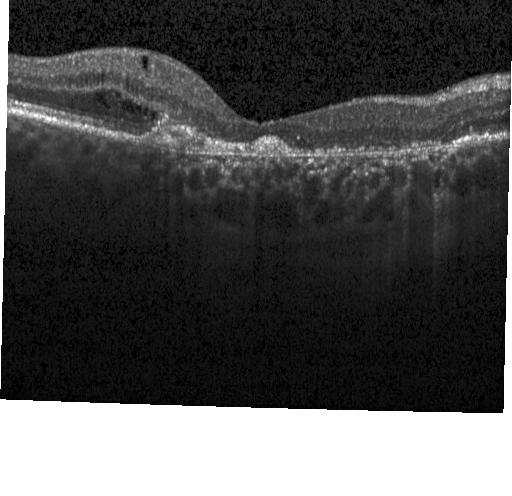 Spectral-domain OCT · optical coherence tomography scan · through the macula · instrument: Heidelberg Spectralis — Finding: choroidal neovascularization (CNV).